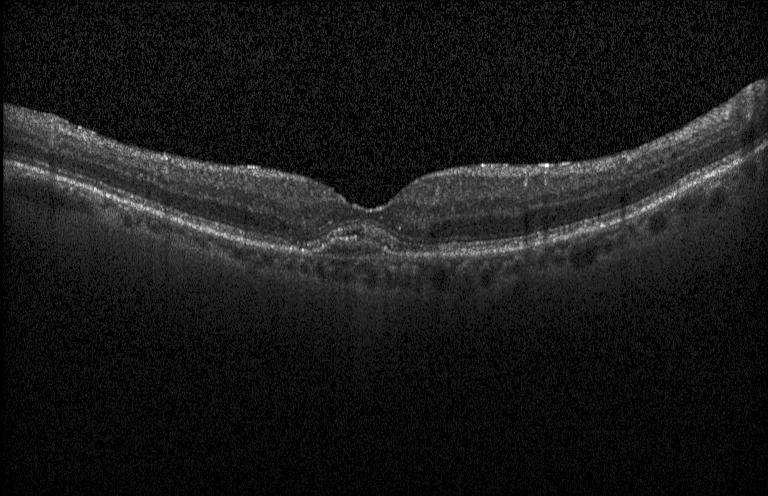
Acquired on a Heidelberg Spectralis. Spectral-domain optical coherence tomography. OCT B-scan. Macular OCT: a choroidal neovascular membrane.